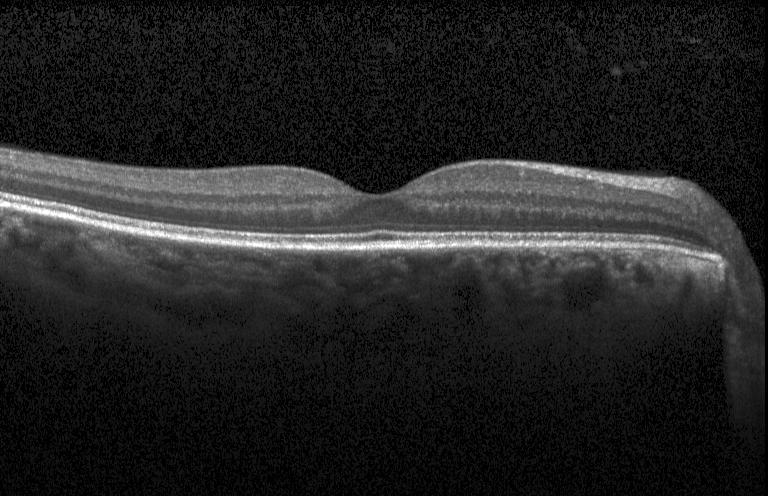 OCT line scan, instrument: Heidelberg Spectralis, fovea-centered
This B-scan demonstrates neither CNV, DME, nor drusen.